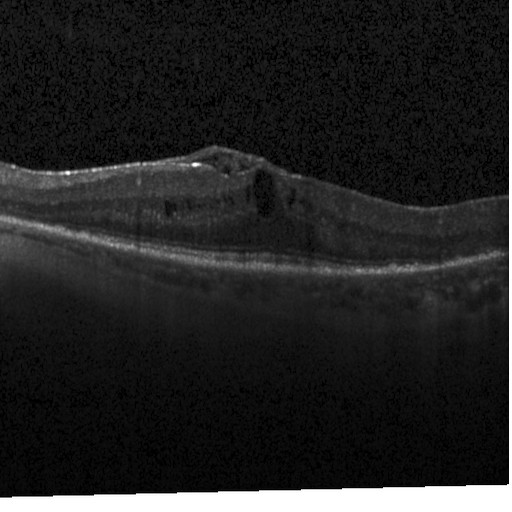 The scan shows diabetic macular edema (DME).